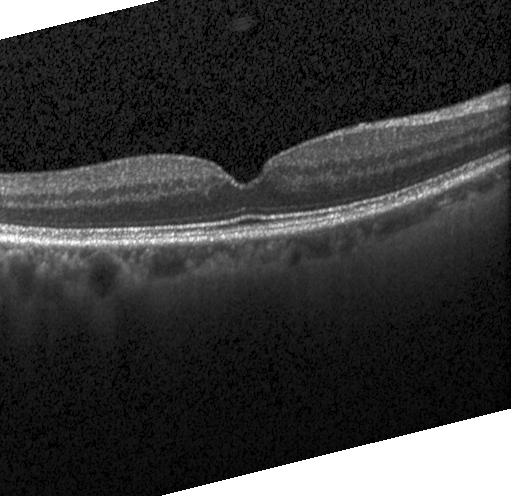

Macular scan; retinal OCT B-scan; SD-OCT.
OCT finding: no evidence of CNV, DME, or drusen.